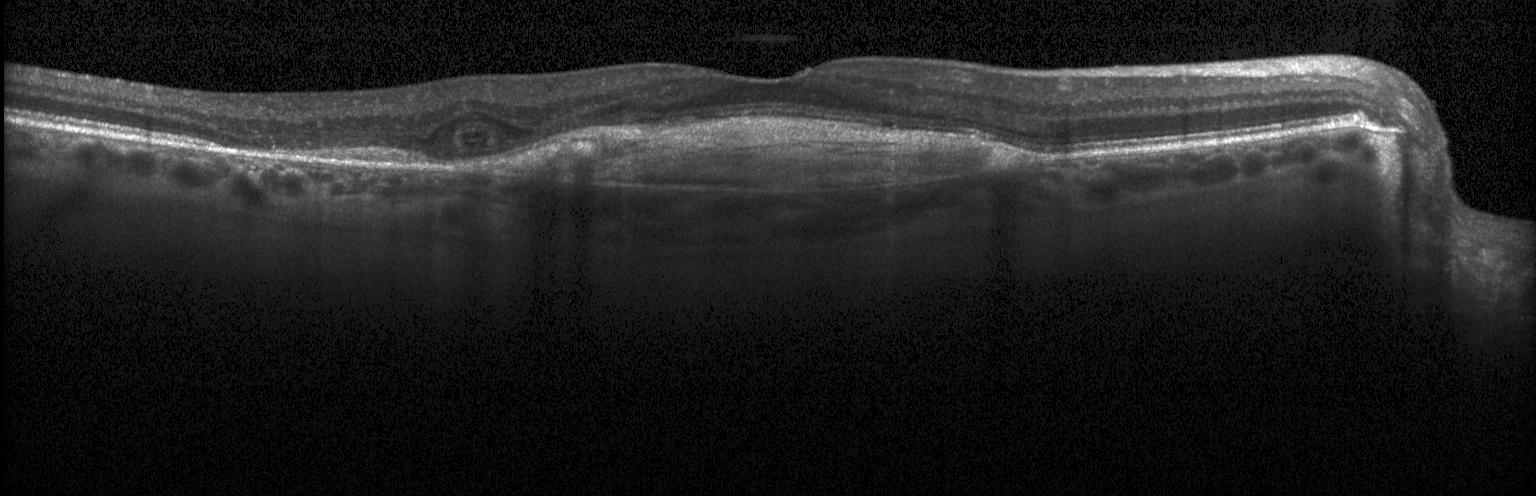 Optical coherence tomography B-scan. Heidelberg Spectralis. Spectral-domain OCT. Fovea-centered
The scan shows CNV.